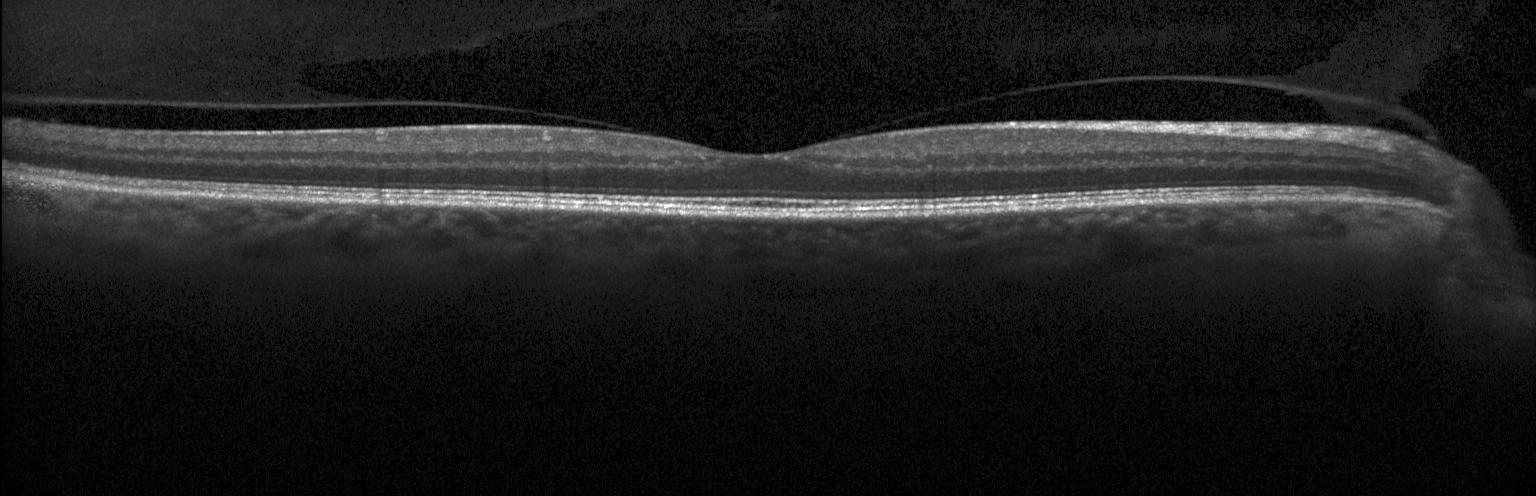

Macular scan · retinal OCT cross-section · SD-OCT.
Finding: no evidence of CNV, DME, or drusen.